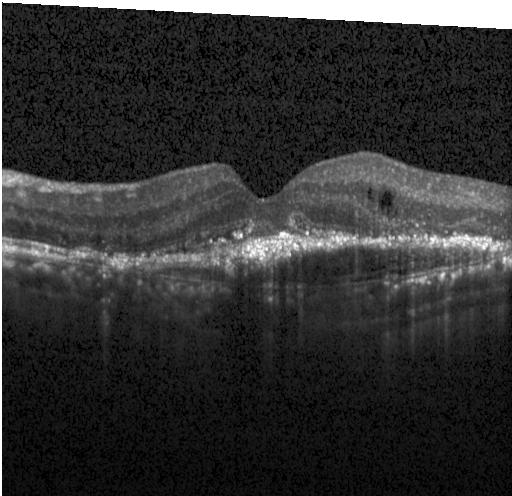
Impression: a choroidal neovascular membrane.